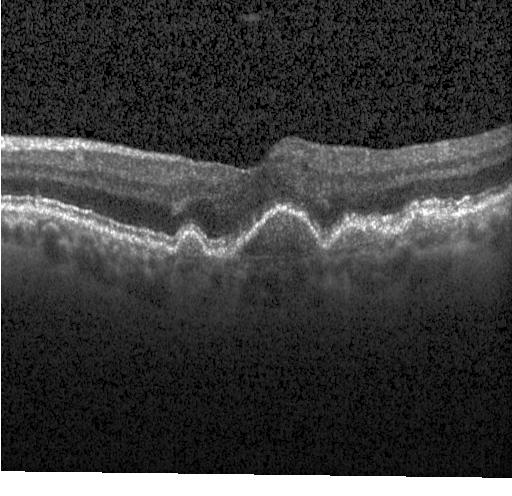
Macular scan, retinal OCT cross-section, spectral-domain optical coherence tomography.
Impression: choroidal neovascularization.